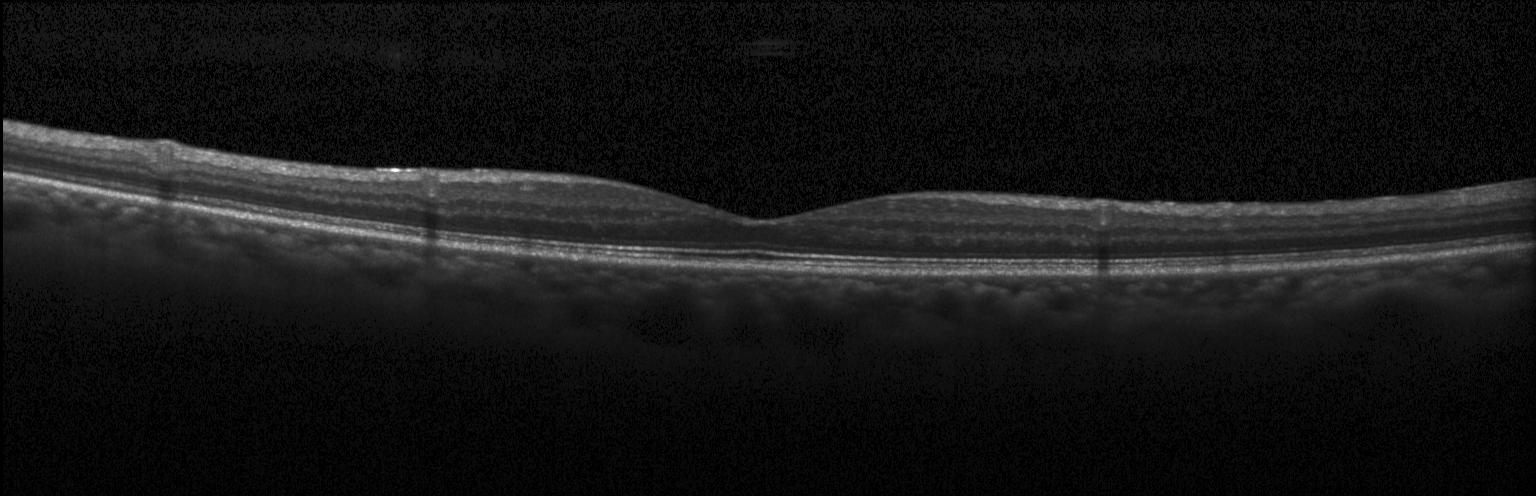
Finding: no evidence of choroidal neovascularization, diabetic macular edema, or drusen.